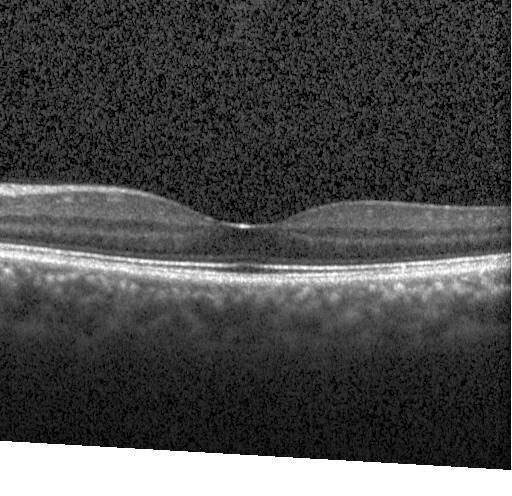
Diagnosis: no choroidal neovascularization, diabetic macular edema, or drusen.